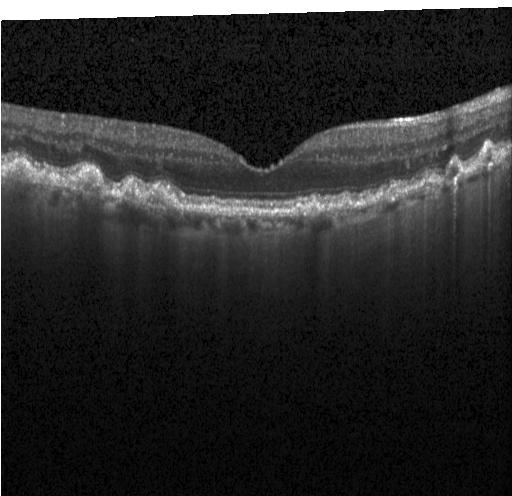

Optical coherence tomography scan, through the macula.
Macular OCT: drusen.